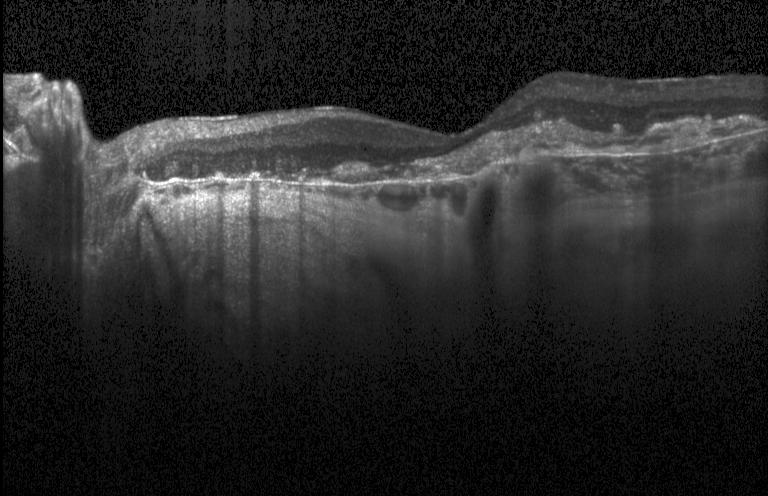 Impression: choroidal neovascularization.